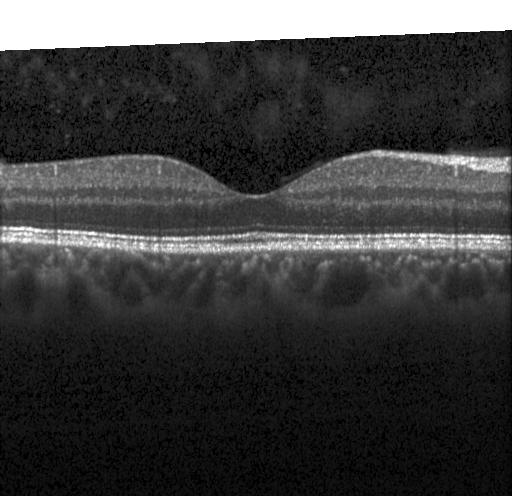
The scan shows no choroidal neovascularization, diabetic macular edema, or drusen.